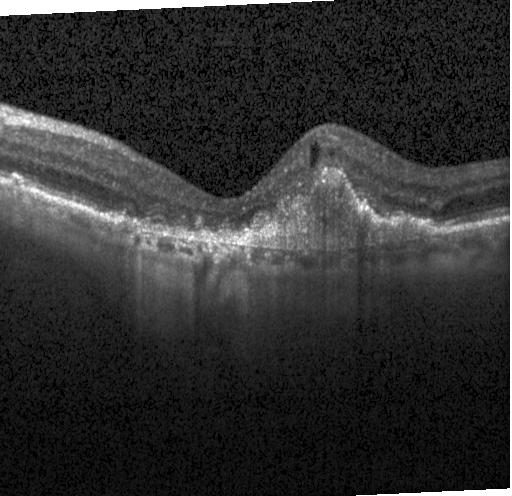
Instrument: Heidelberg Spectralis · through the macula · OCT B-scan · SD-OCT
Macular OCT: a choroidal neovascular membrane.